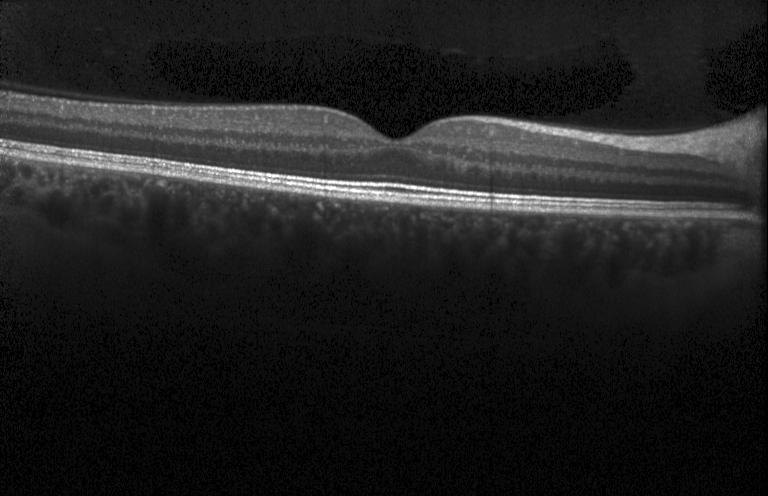
Macular OCT: no CNV, no DME, and no drusen.